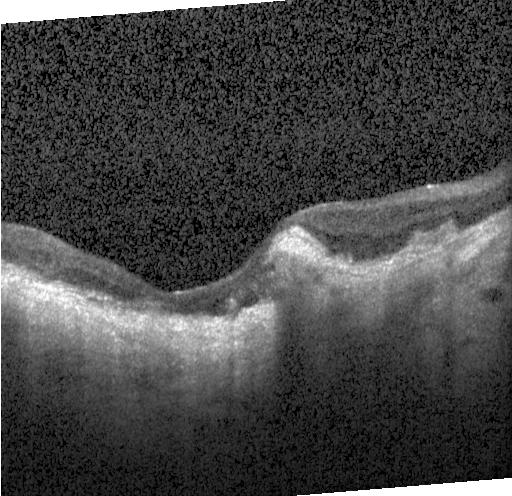 Optical coherence tomography scan.
Finding: a choroidal neovascular membrane.